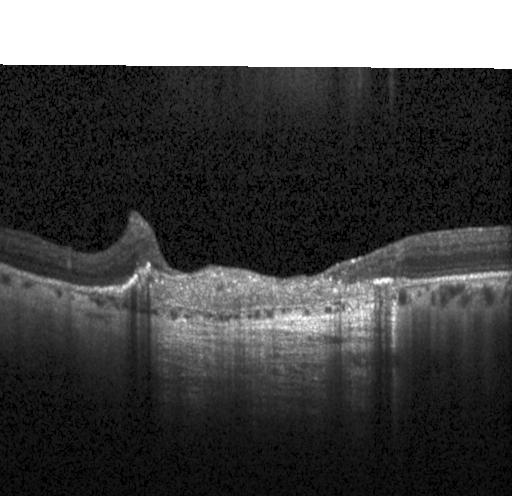 Retinal OCT B-scan, spectral-domain optical coherence tomography, Heidelberg Spectralis OCT system — Impression: choroidal neovascularization.